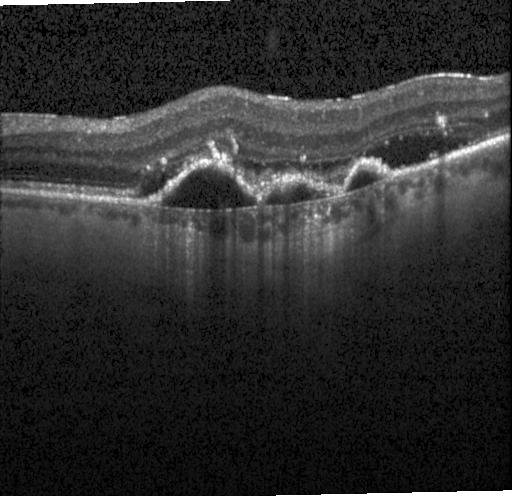 Heidelberg Spectralis OCT system · optical coherence tomography B-scan · centered on the fovea · spectral-domain optical coherence tomography. OCT finding: a choroidal neovascular membrane.